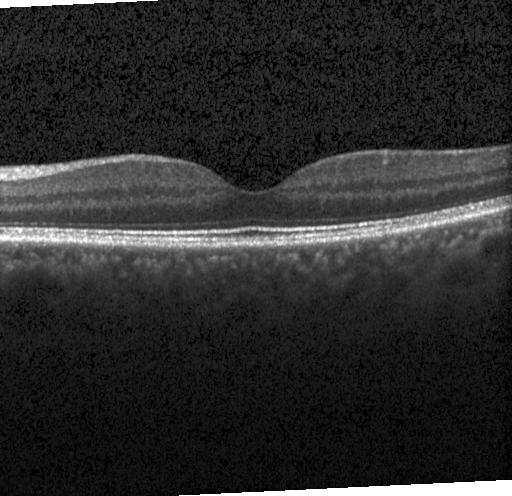
OCT B-scan. Diagnosis: no evidence of CNV, DME, or drusen.